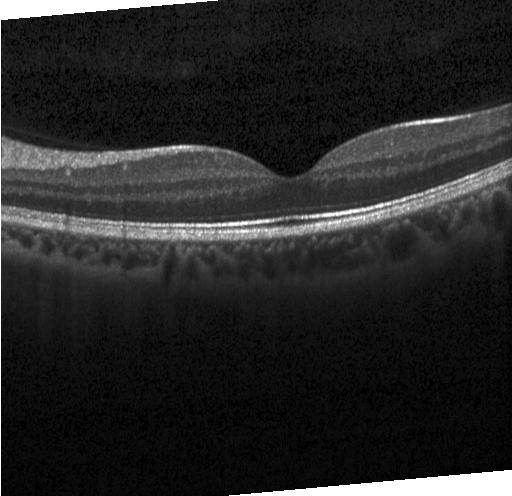

No CNV, no DME, and no drusen.